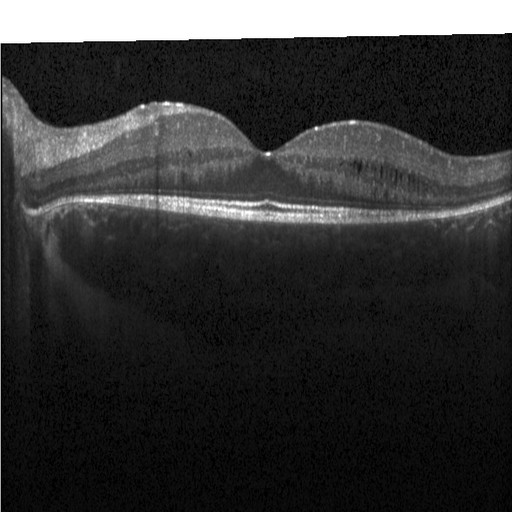
Diagnosis: diabetic macular edema.